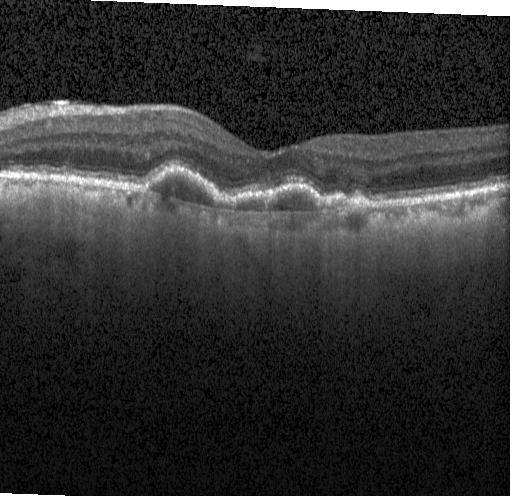 Instrument: Heidelberg Spectralis; retinal OCT B-scan; SD-OCT. Dx: a choroidal neovascular membrane.